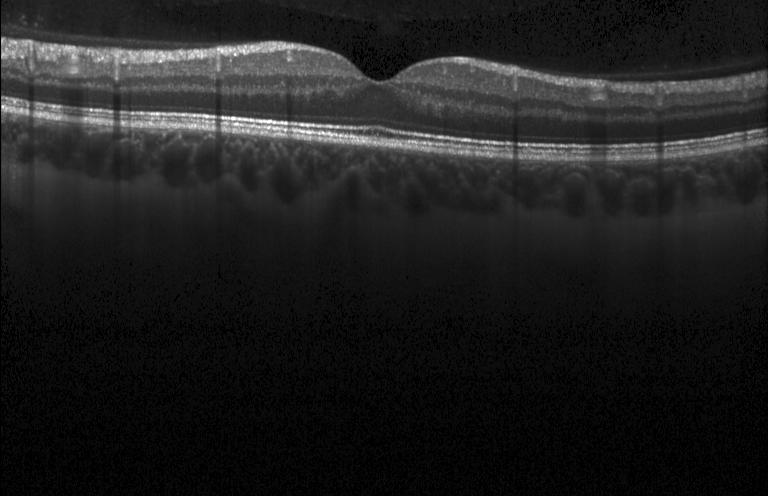 Retinal OCT cross-section showing no CNV, no DME, and no drusen.